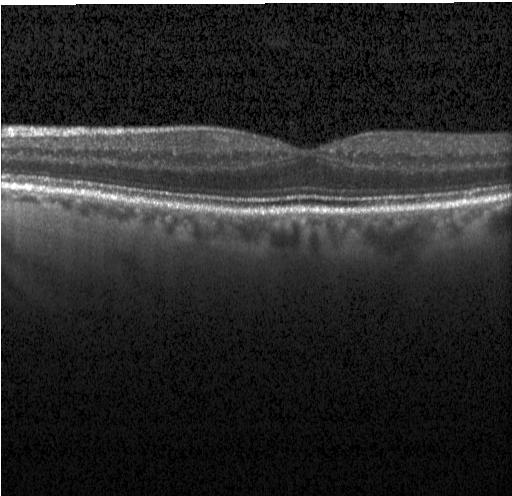

Retinal OCT cross-section, SD-OCT.
The scan shows no choroidal neovascularization, no diabetic macular edema, and no drusen.